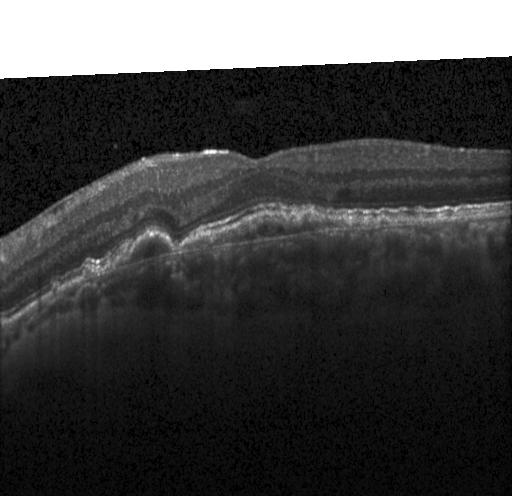
Diagnosis: choroidal neovascularization (CNV).